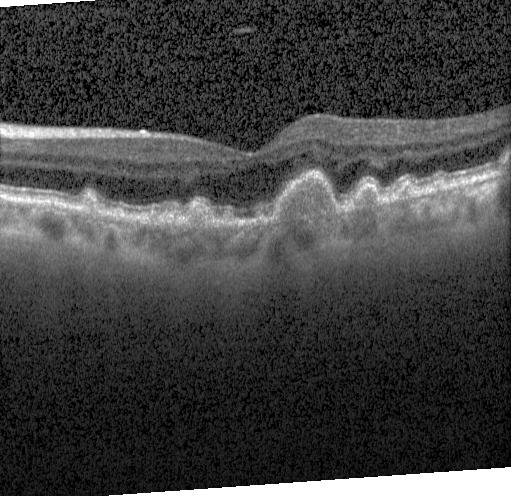 The scan shows sub-RPE drusenoid deposits.